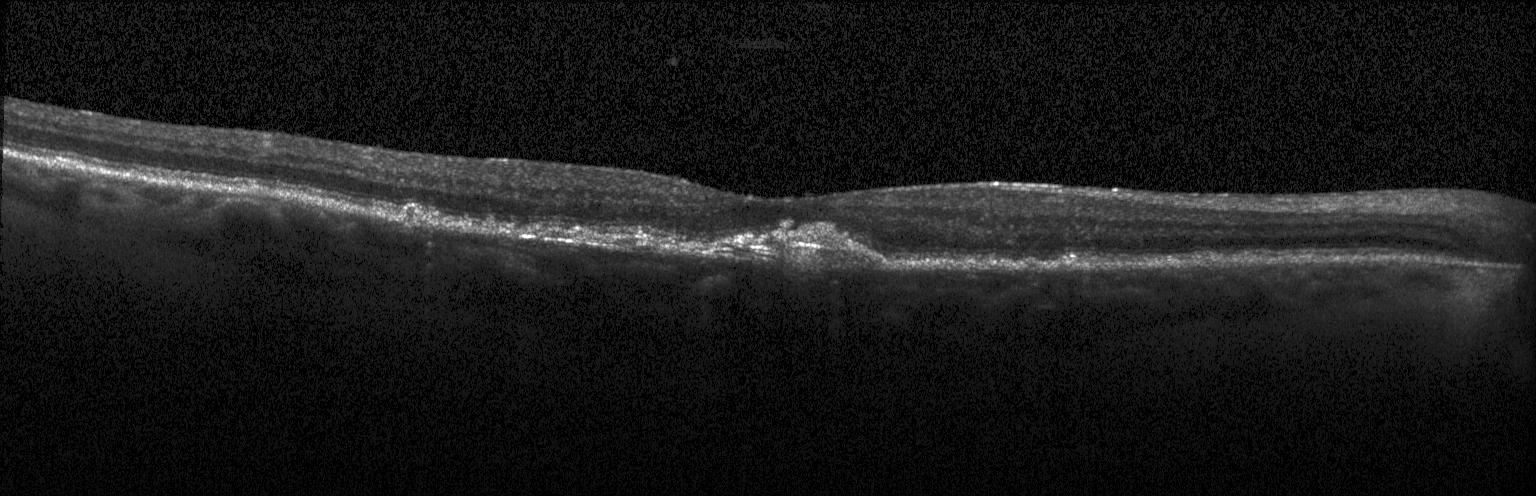
OCT B-scan showing CNV.